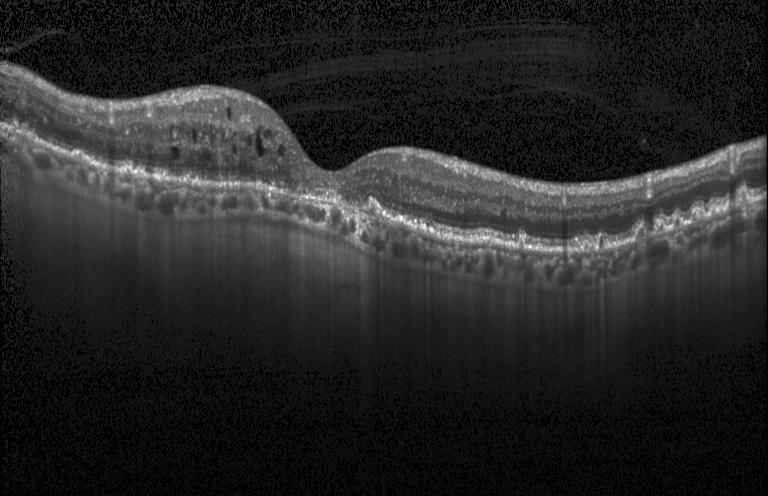
OCT B-scan showing a choroidal neovascular membrane.